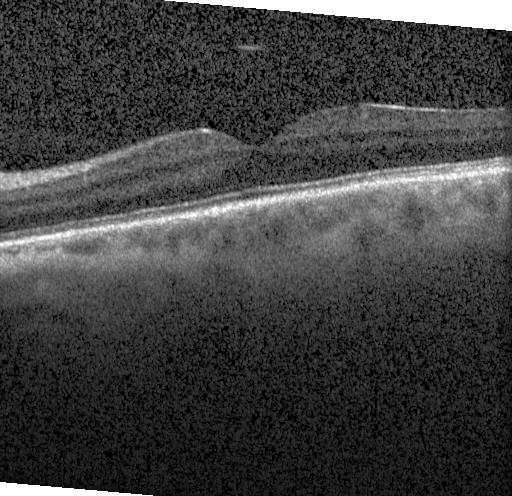
Impression: no CNV, DME, or drusen.